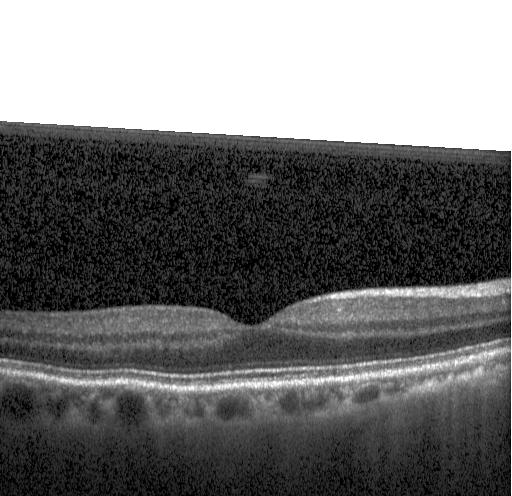 Dx: no CNV, no DME, and no drusen.